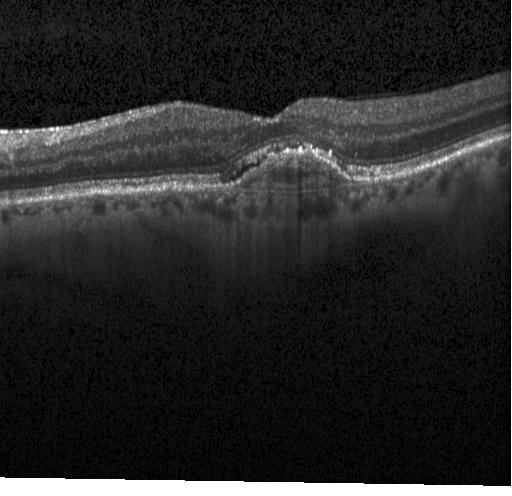 The scan shows CNV.